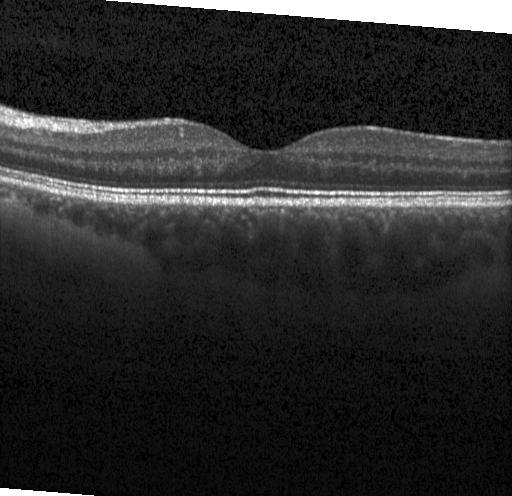 Macular scan · optical coherence tomography B-scan.
Finding: neither choroidal neovascularization, diabetic macular edema, nor drusen.